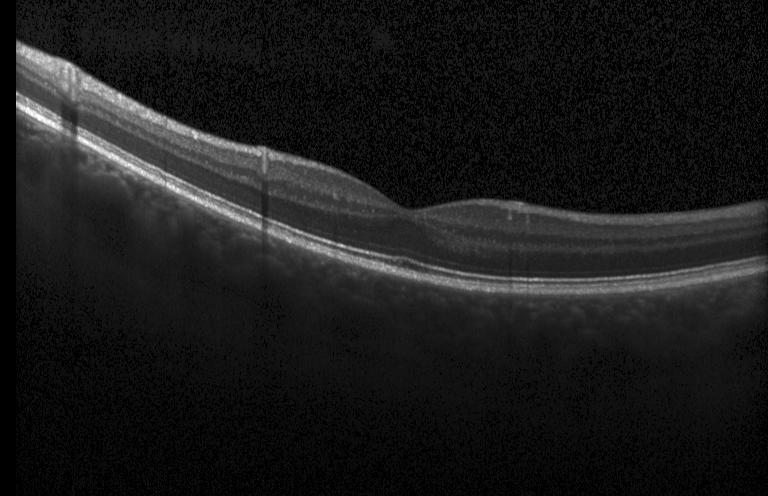

OCT finding: no evidence of choroidal neovascularization, diabetic macular edema, or drusen.